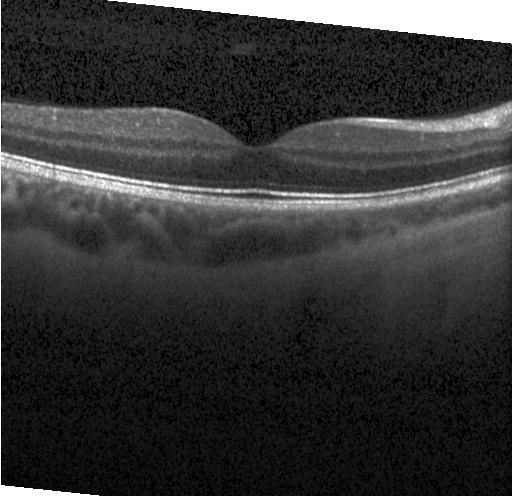
Heidelberg Spectralis OCT system · retinal OCT cross-section · spectral-domain optical coherence tomography · through the macula. Finding: neither choroidal neovascularization, diabetic macular edema, nor drusen.